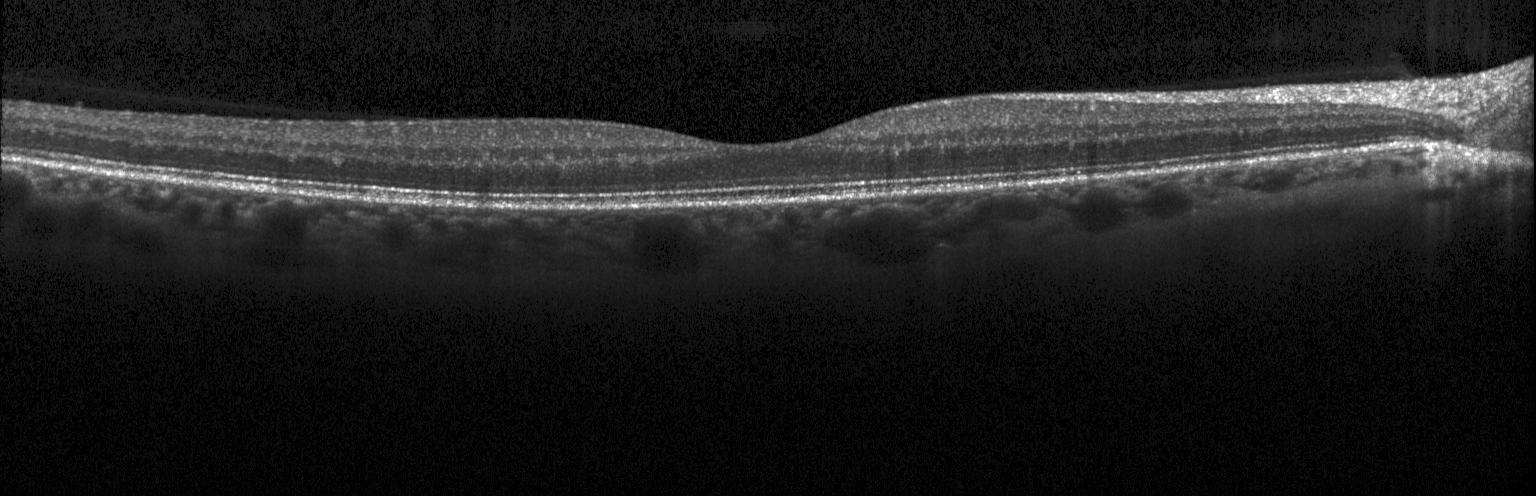 Assessment: no CNV, no DME, and no drusen.